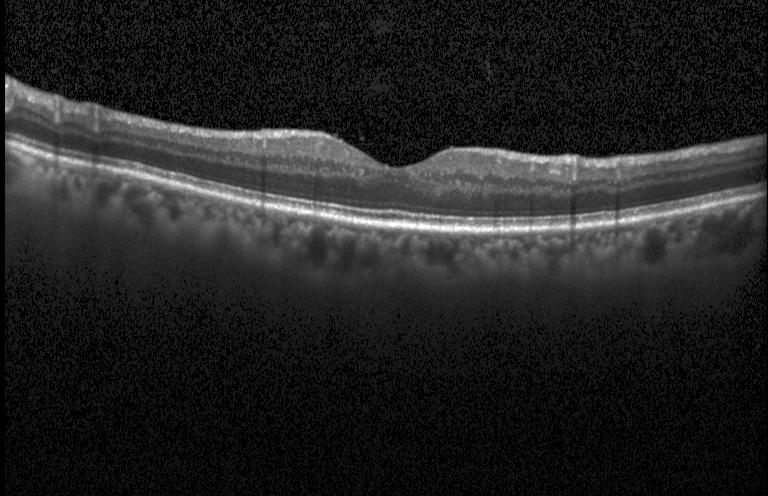

Horizontal scan through the fovea. OCT line scan — Finding: no choroidal neovascularization, no diabetic macular edema, and no drusen.